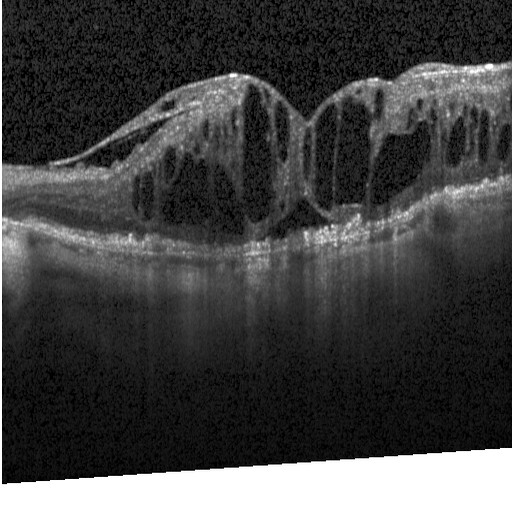
Retinal OCT B-scan. SD-OCT.
Finding: diabetic macular edema (DME).